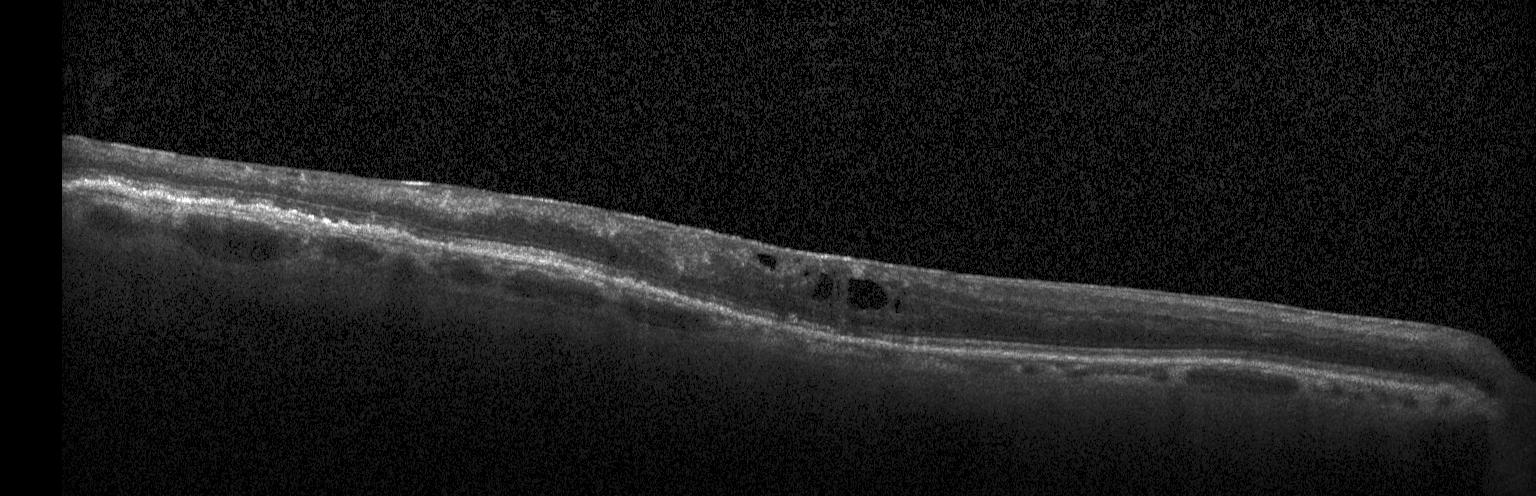
Retinal OCT B-scan; Heidelberg Spectralis; fovea-centered
Diagnosis: CNV.